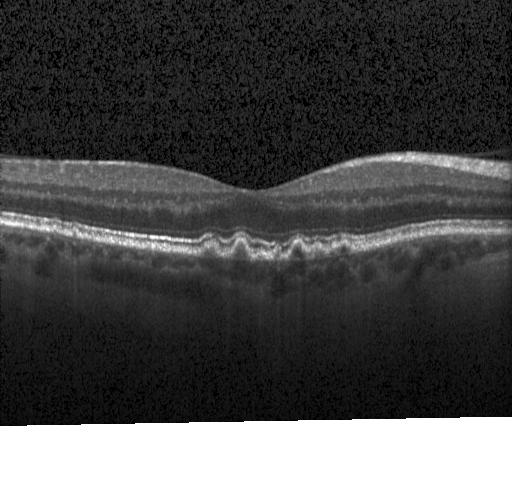
Impression: drusen.